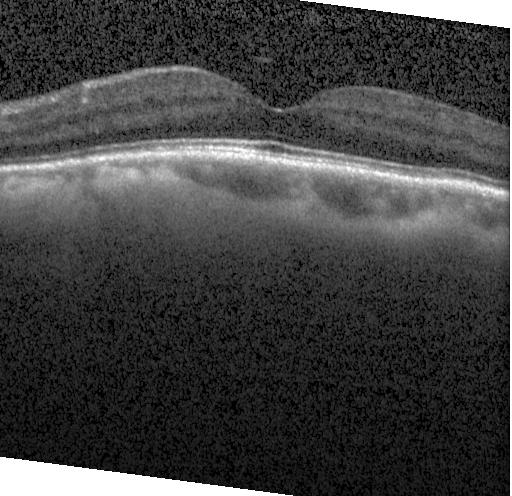 No CNV, DME, or drusen.